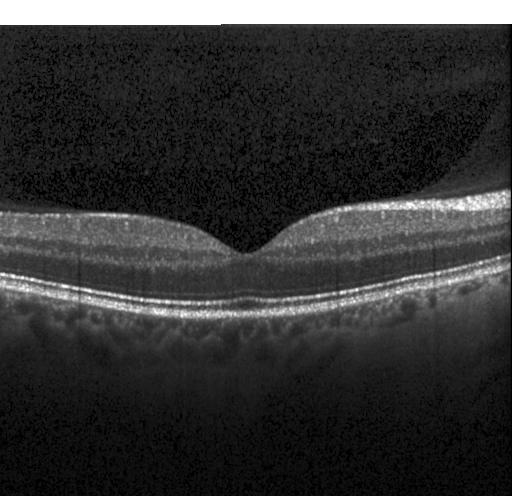 Impression: no choroidal neovascularization, diabetic macular edema, or drusen.